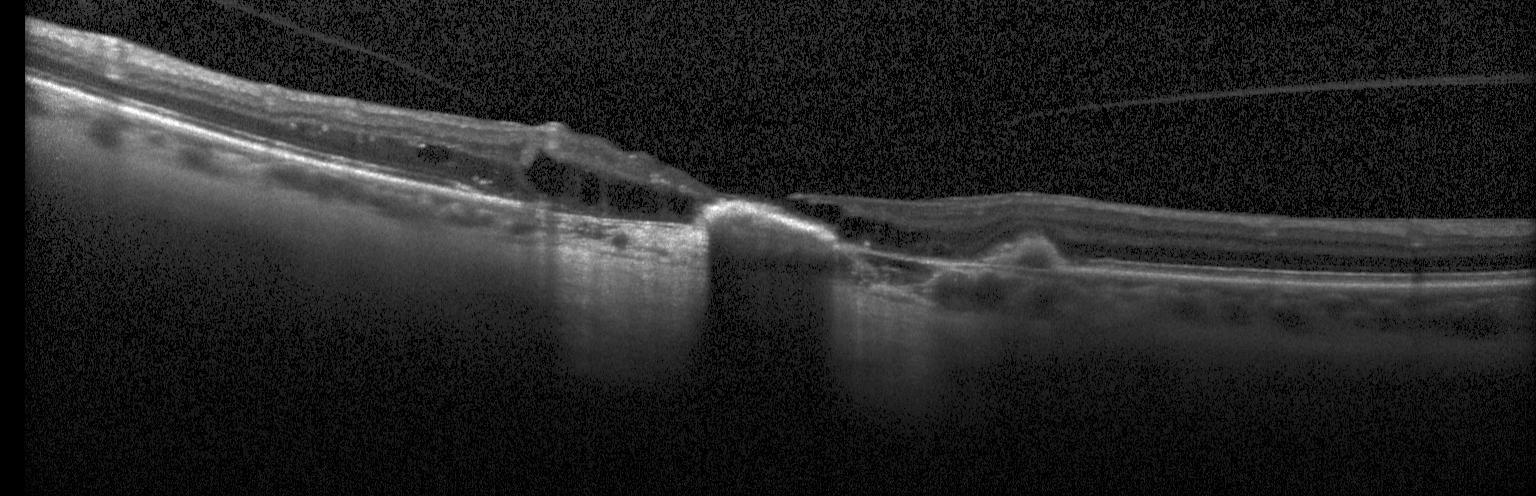
OCT B-scan.
Impression: a choroidal neovascular membrane.